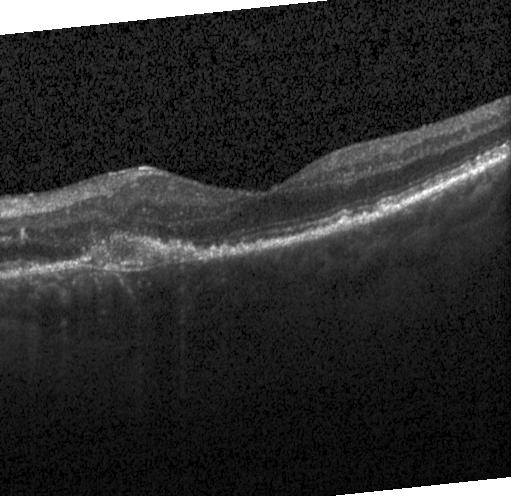 OCT line scan; spectral-domain optical coherence tomography; Heidelberg Spectralis OCT system; through the macula
Impression: choroidal neovascularization.